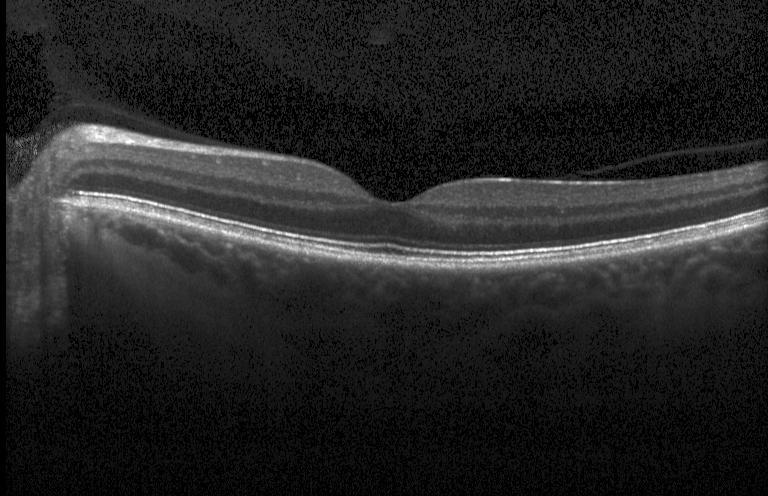
Optical coherence tomography B-scan — Impression: neither choroidal neovascularization, diabetic macular edema, nor drusen.